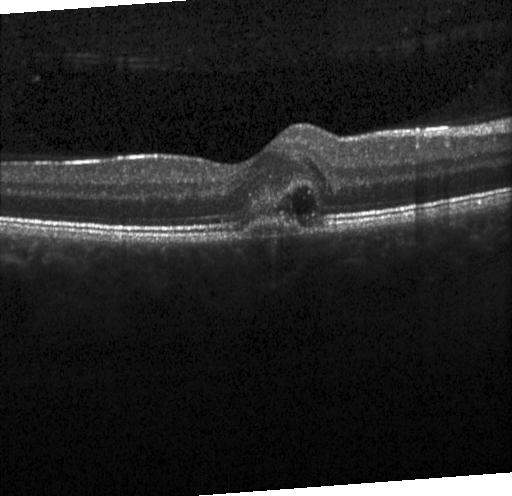 Macular OCT: choroidal neovascularization (CNV).